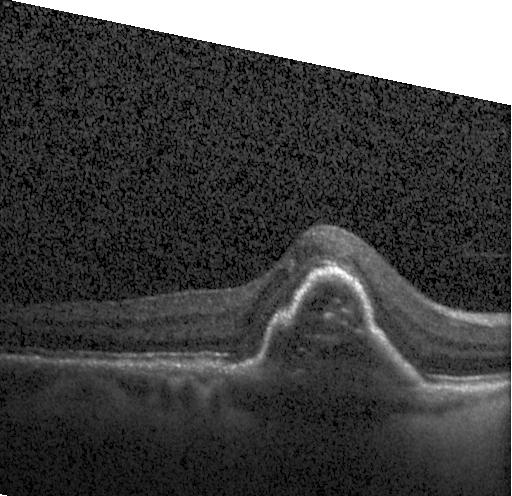
Impression: a choroidal neovascular membrane.